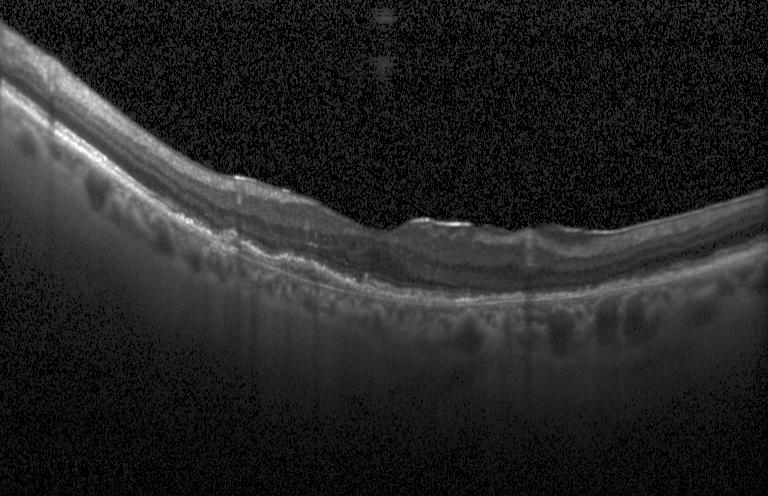
Spectral-domain optical coherence tomography; optical coherence tomography B-scan.
Choroidal neovascularization.